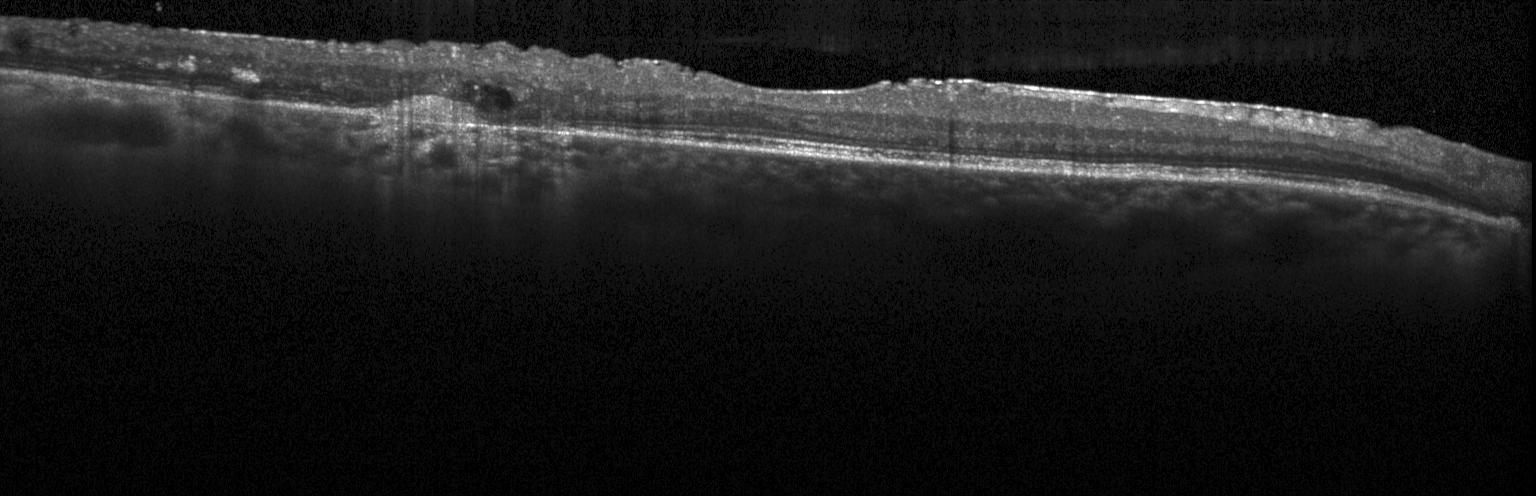 Horizontal scan through the fovea; acquired on a Heidelberg Spectralis; OCT line scan
Assessment: a choroidal neovascular membrane.